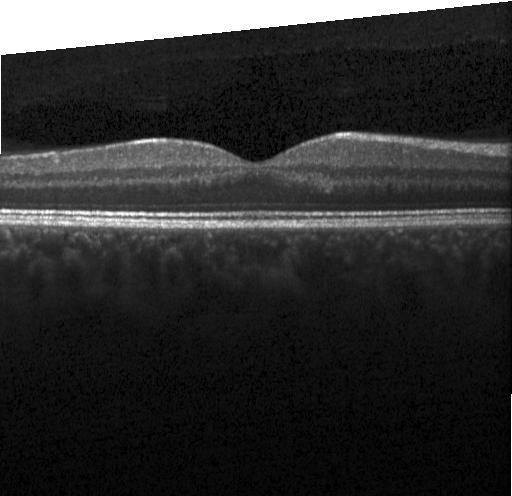
Spectral-domain OCT, acquired on a Heidelberg Spectralis, OCT B-scan — OCT finding: no CNV, no DME, and no drusen.